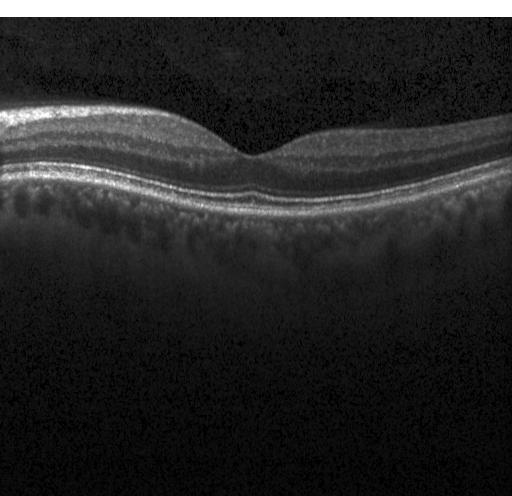

Retinal OCT cross-section.
Finding: neither choroidal neovascularization, diabetic macular edema, nor drusen.